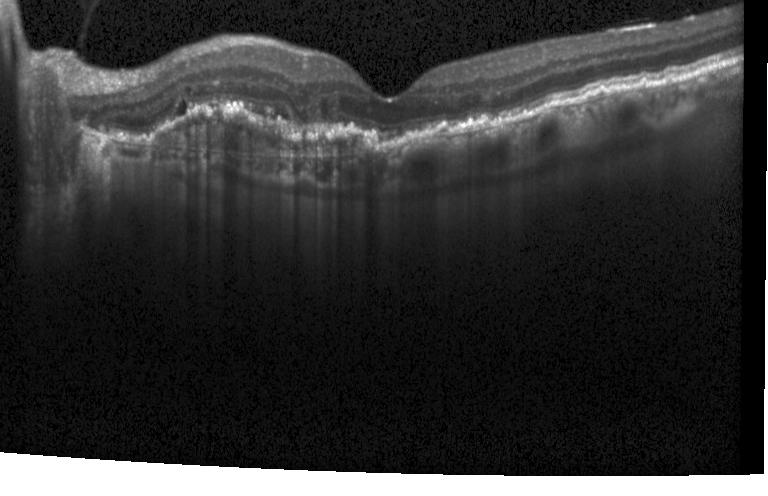 Heidelberg Spectralis · optical coherence tomography scan.
Diagnosis: choroidal neovascularization (CNV).